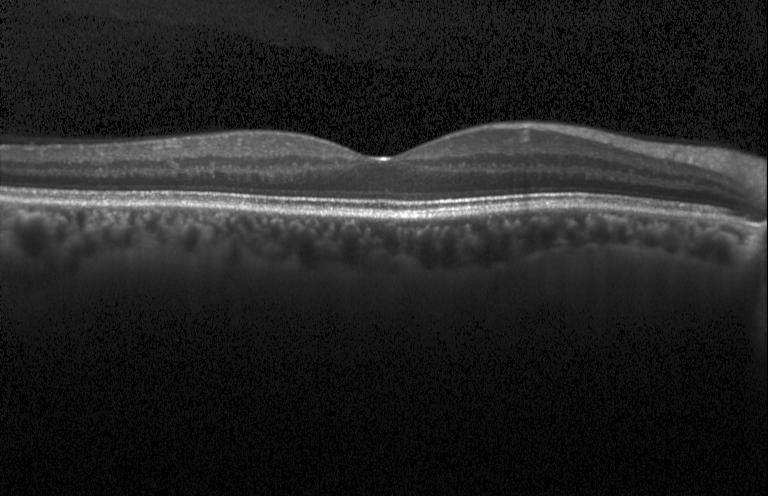
Assessment: no evidence of choroidal neovascularization, diabetic macular edema, or drusen.